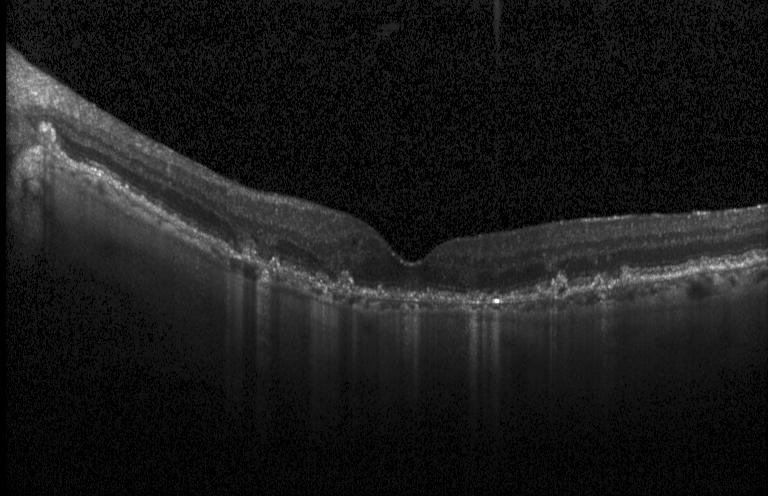
Retinal OCT B-scan — Diagnosis: CNV.